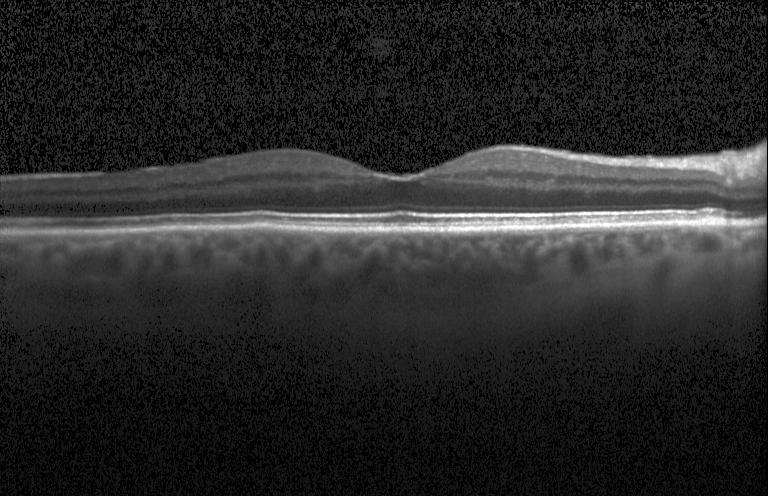

Optical coherence tomography scan.
Impression: no evidence of choroidal neovascularization, diabetic macular edema, or drusen.